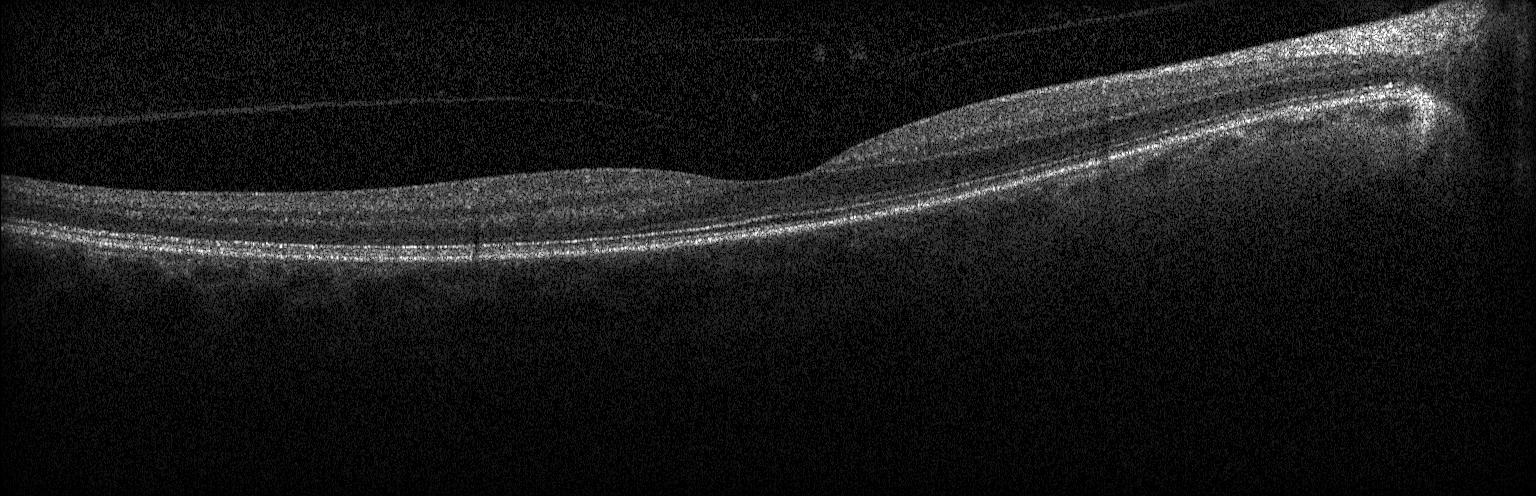
Macular scan · SD-OCT · optical coherence tomography B-scan · Heidelberg Spectralis.
Macular OCT: no choroidal neovascularization, no diabetic macular edema, and no drusen.